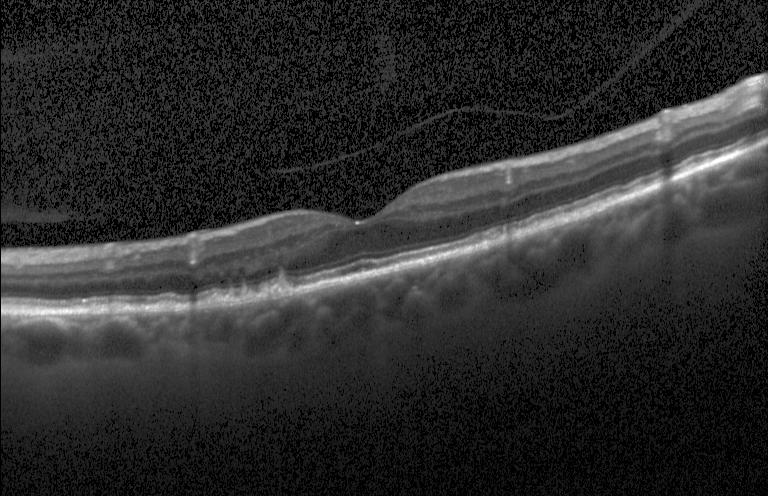

Centered on the fovea, optical coherence tomography B-scan, SD-OCT.
Impression: sub-RPE drusenoid deposits.